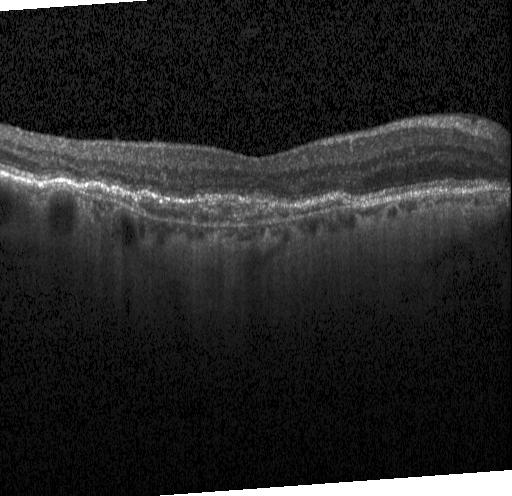

Spectral-domain optical coherence tomography, retinal OCT B-scan, through the macula. Impression: choroidal neovascularization.